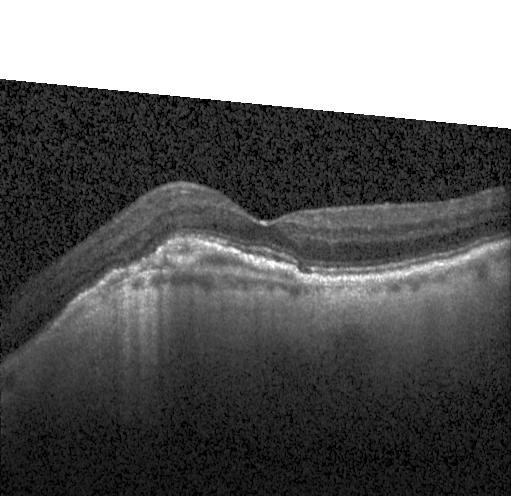
Retinal OCT B-scan. Assessment: a choroidal neovascular membrane.